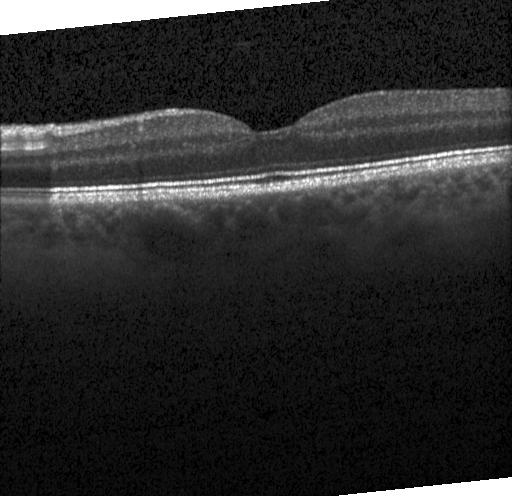 Spectral-domain OCT B-scan: no choroidal neovascularization, no diabetic macular edema, and no drusen.